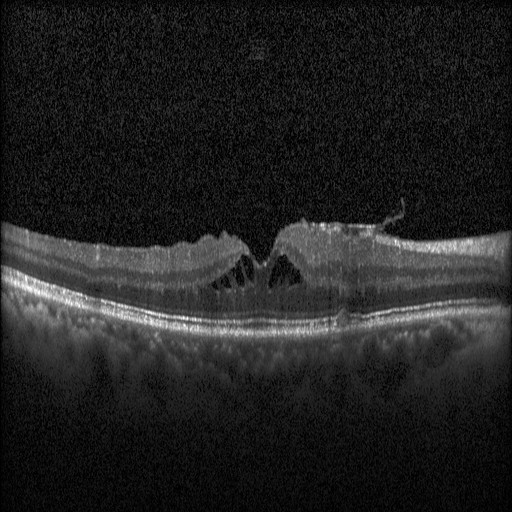

Spectral-domain optical coherence tomography, horizontal scan through the fovea, optical coherence tomography scan, instrument: Heidelberg Spectralis.
Dx: DME.